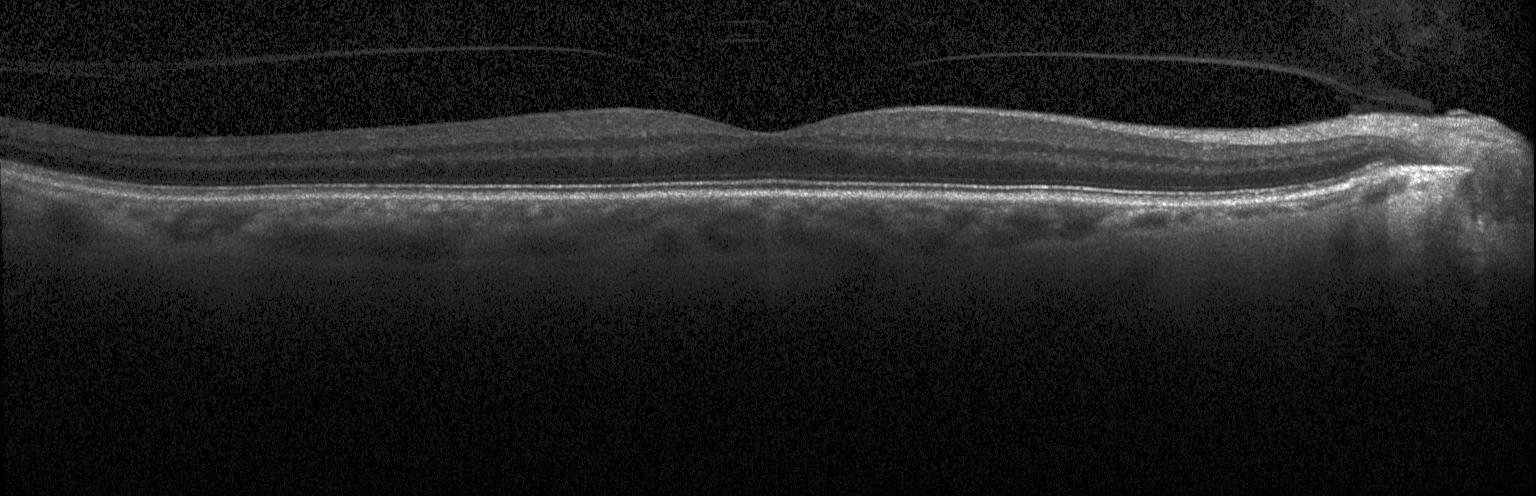
OCT B-scan; SD-OCT. Diagnosis: no evidence of CNV, DME, or drusen.